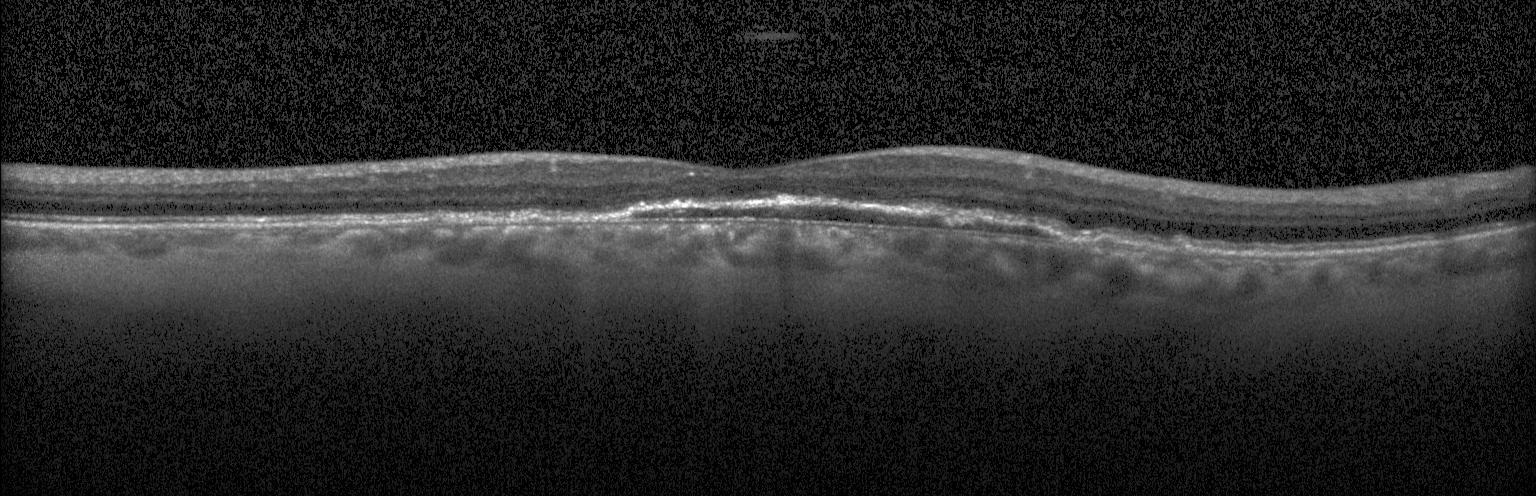 This B-scan demonstrates a choroidal neovascular membrane.